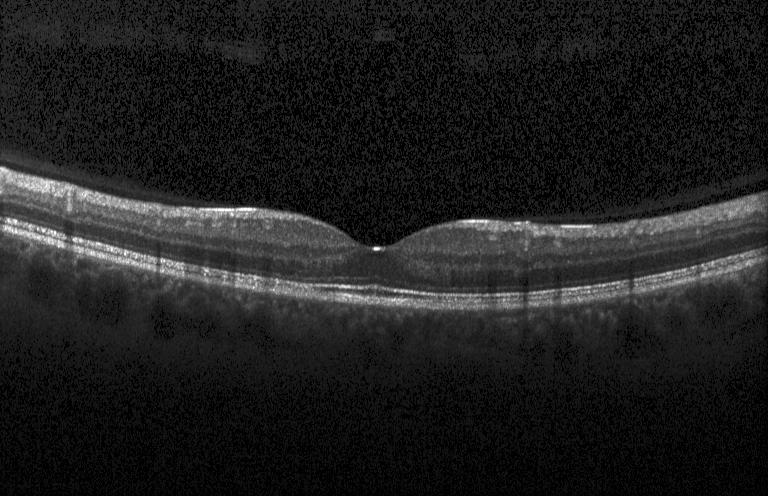
Retinal OCT cross-section
Diagnosis: no choroidal neovascularization, no diabetic macular edema, and no drusen.